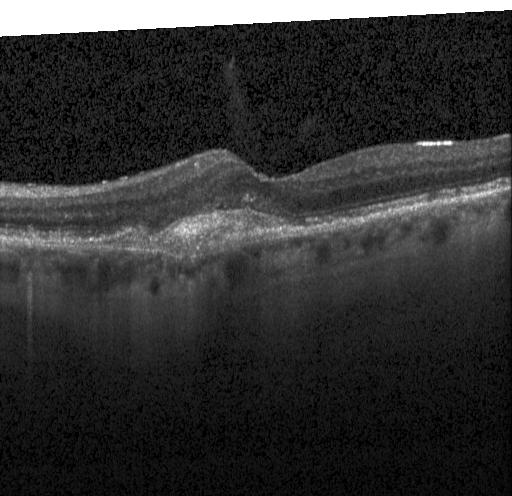
SD-OCT. Instrument: Heidelberg Spectralis. OCT B-scan
This B-scan demonstrates a choroidal neovascular membrane.